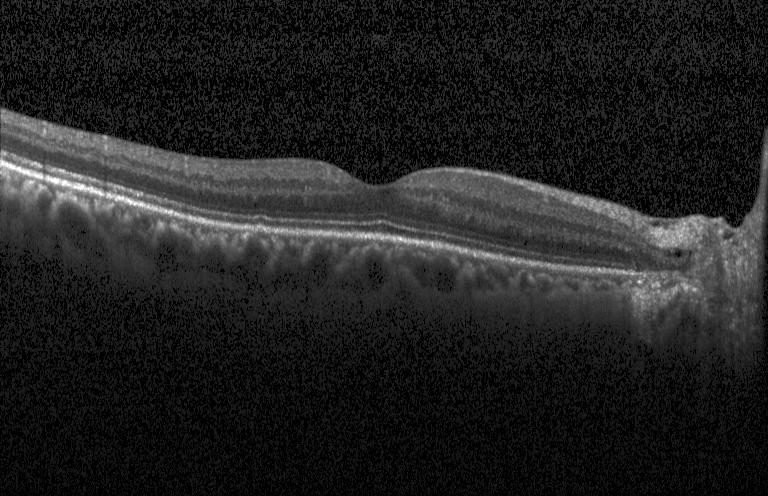

Macular scan, retinal OCT cross-section — The scan shows no CNV, DME, or drusen.